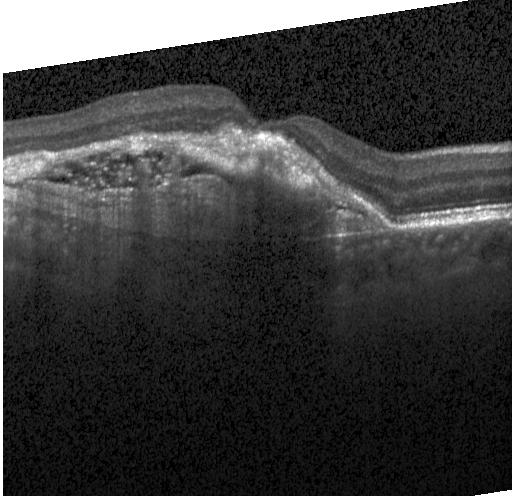
Macular OCT: a choroidal neovascular membrane.